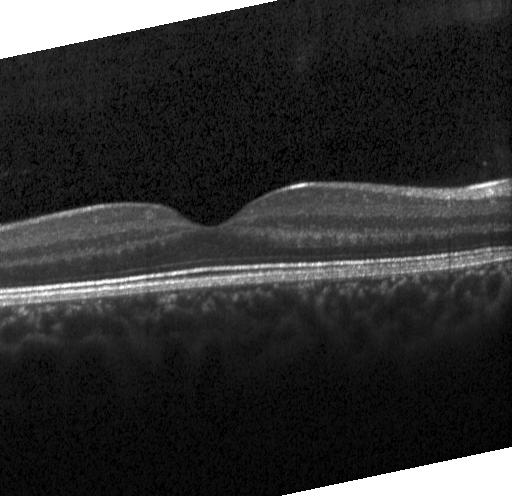

Optical coherence tomography scan · centered on the fovea · spectral-domain optical coherence tomography · Heidelberg Spectralis. Impression: no evidence of CNV, DME, or drusen.